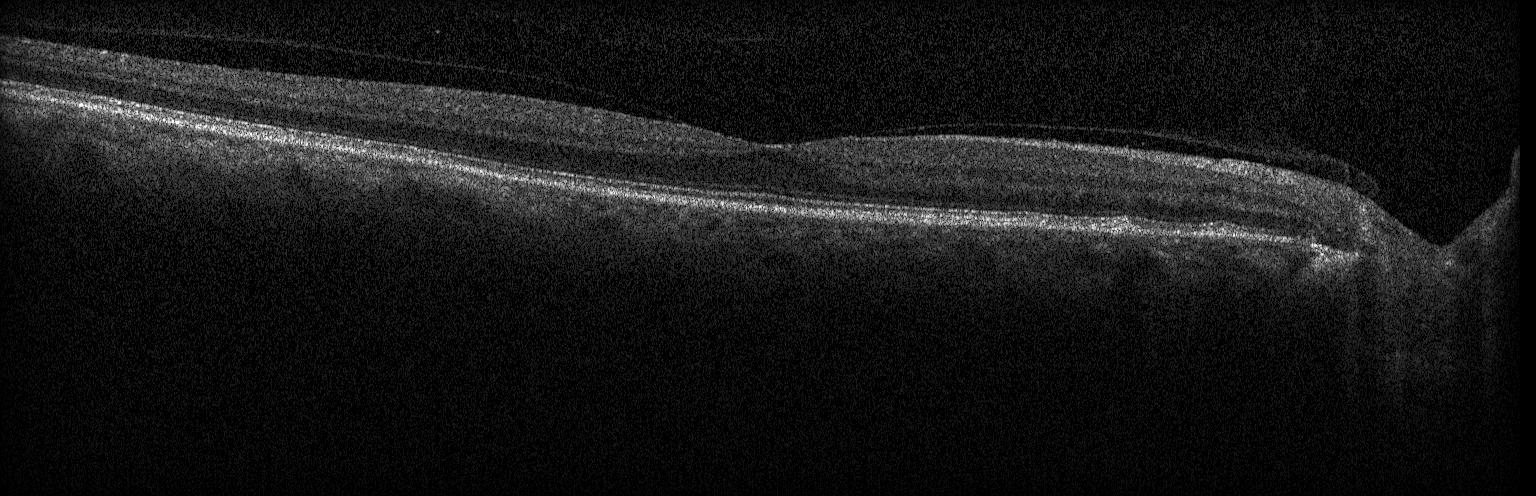
The scan shows no choroidal neovascularization, diabetic macular edema, or drusen.